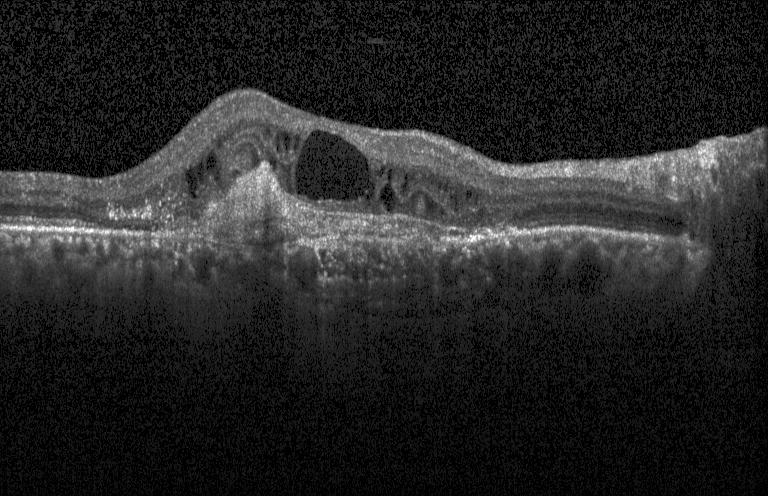

Centered on the fovea, optical coherence tomography scan, spectral-domain optical coherence tomography, Heidelberg Spectralis OCT system
Finding: a choroidal neovascular membrane.